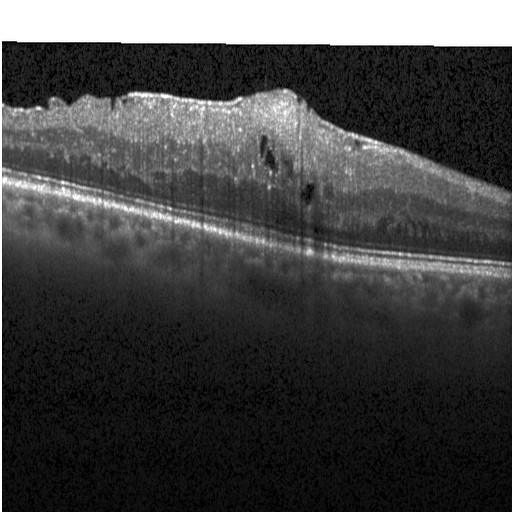

Impression: DME.